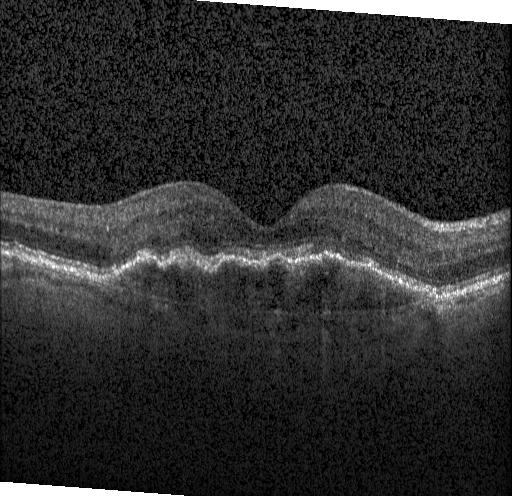 Optical coherence tomography scan. Macular OCT: choroidal neovascularization.